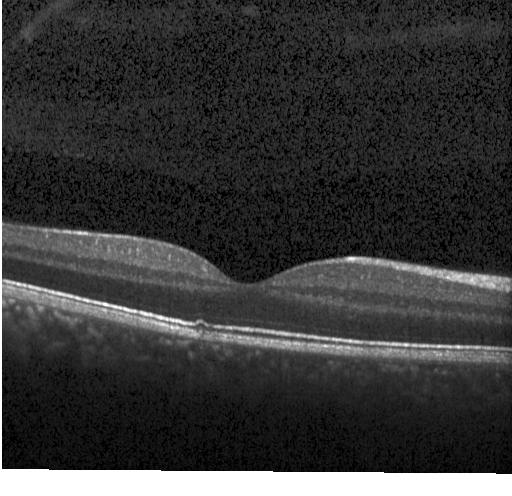 Dx: multiple drusen.